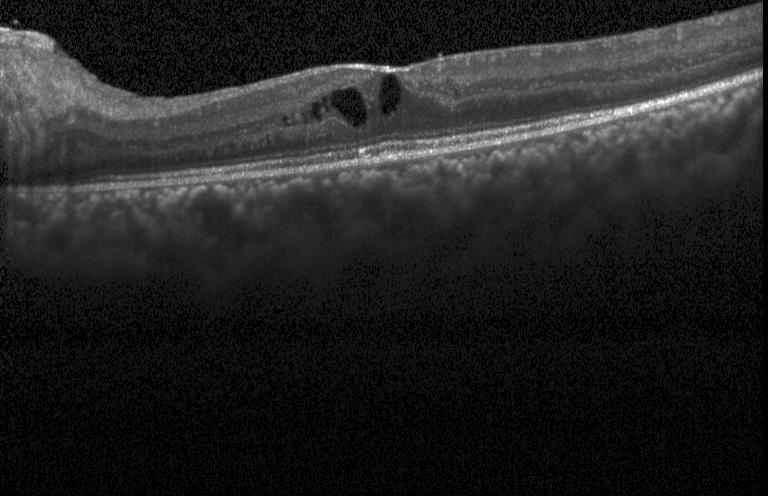

Optical coherence tomography B-scan. Macular scan
Diagnosis: diabetic macular edema.